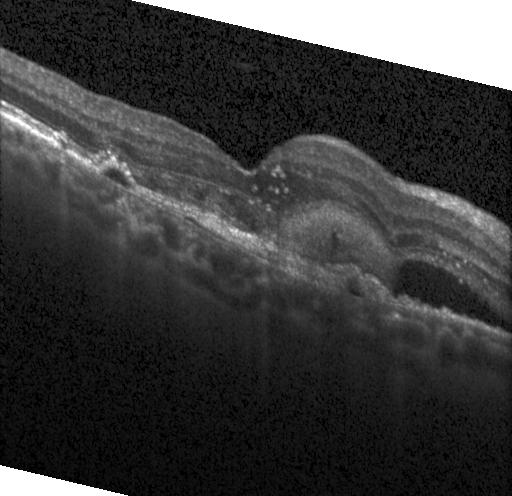
Macular OCT: a choroidal neovascular membrane.